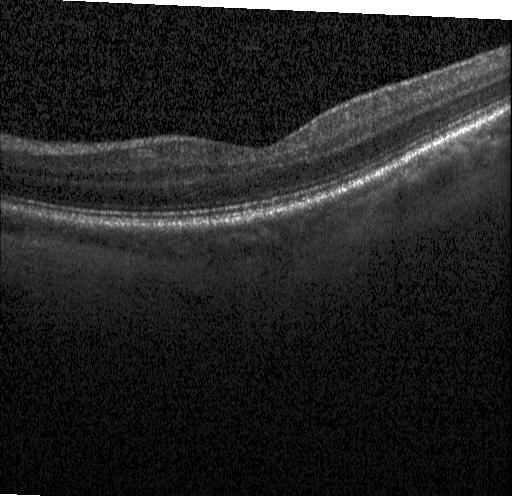
Diagnosis: neither CNV, DME, nor drusen.